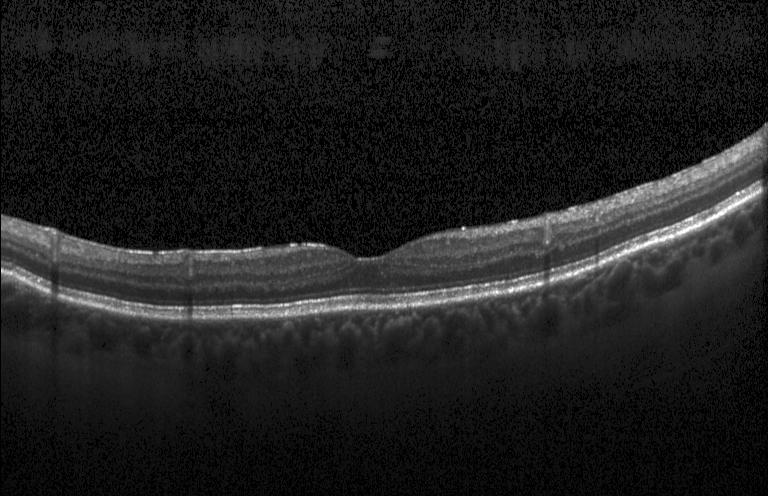 Dx: no CNV, no DME, and no drusen.